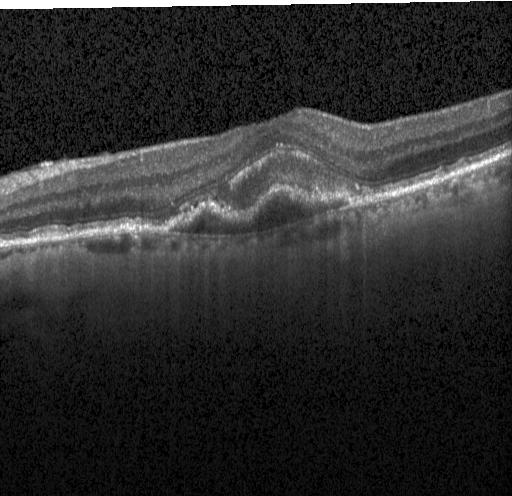 SD-OCT, instrument: Heidelberg Spectralis, centered on the fovea, optical coherence tomography B-scan — Finding: a choroidal neovascular membrane.